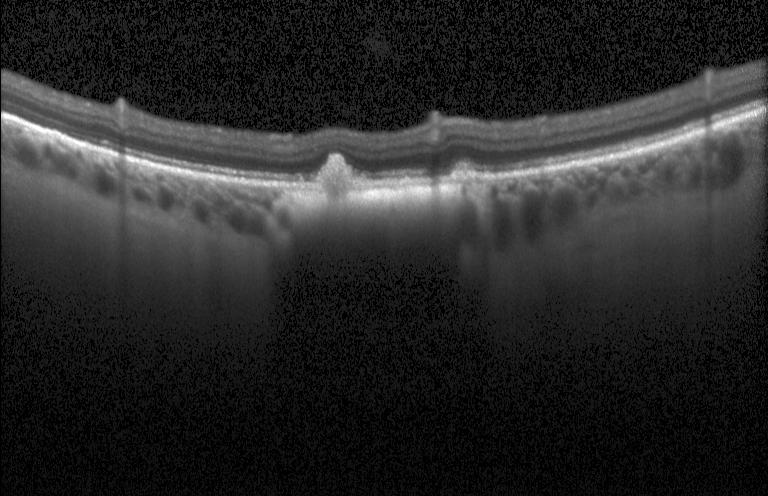
Retinal OCT cross-section showing choroidal neovascularization (CNV).